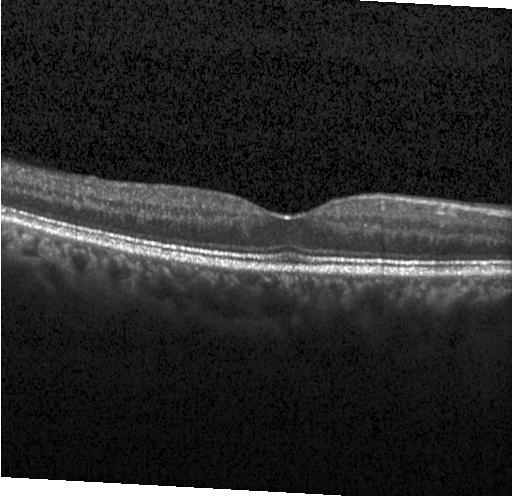
OCT B-scan showing no choroidal neovascularization, no diabetic macular edema, and no drusen.